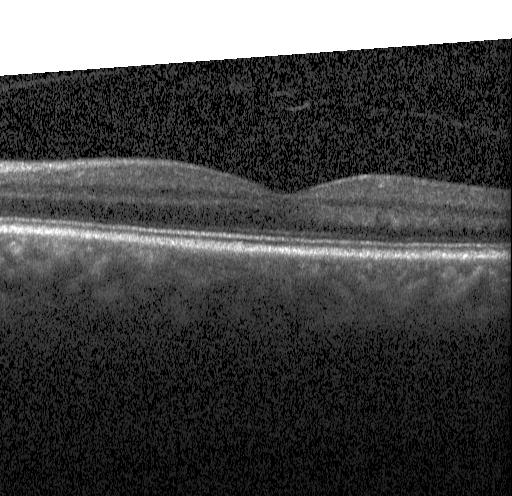
OCT B-scan. Diagnosis: no choroidal neovascularization, diabetic macular edema, or drusen.